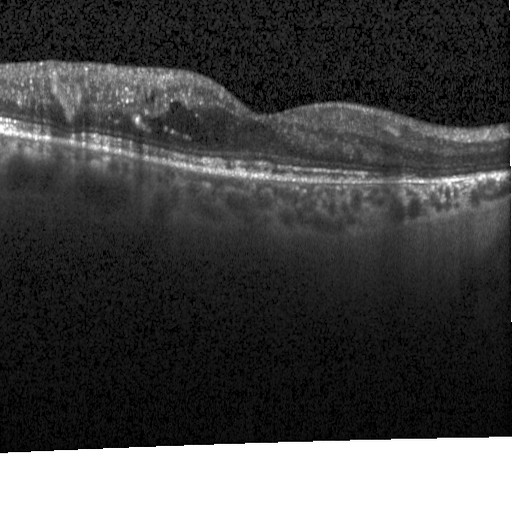

Through the macula, OCT line scan — Macular OCT: DME.